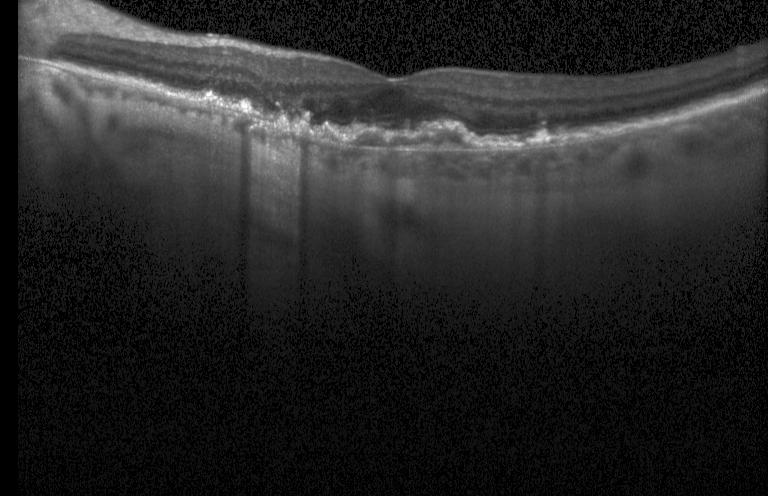 OCT B-scan. Assessment: choroidal neovascularization.